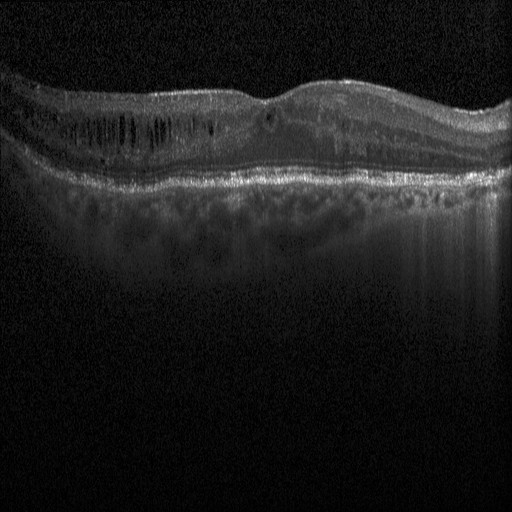
Spectral-domain OCT B-scan: DME.